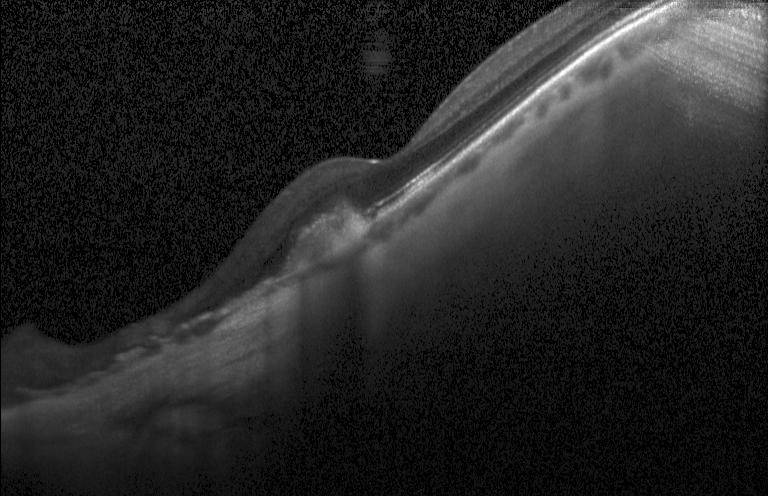 Horizontal scan through the fovea · spectral-domain optical coherence tomography · acquired on a Heidelberg Spectralis · OCT B-scan
Diagnosis: choroidal neovascularization (CNV).